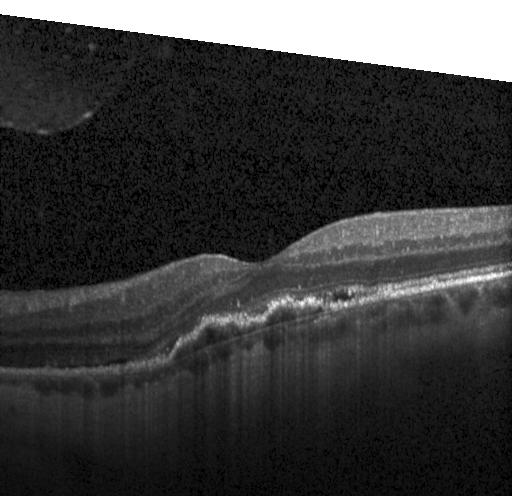 Optical coherence tomography B-scan.
Diagnosis: a choroidal neovascular membrane.